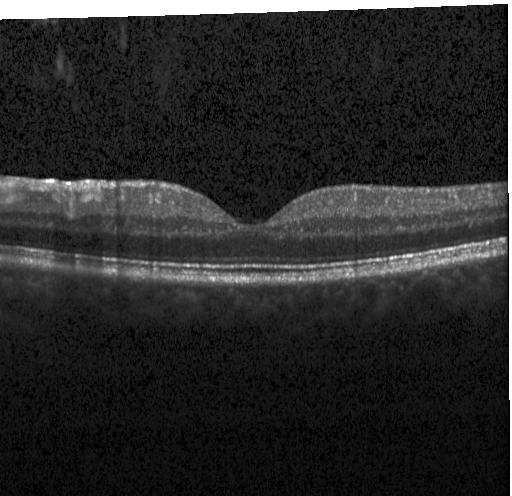

Retinal OCT B-scan
Diagnosis: no evidence of choroidal neovascularization, diabetic macular edema, or drusen.